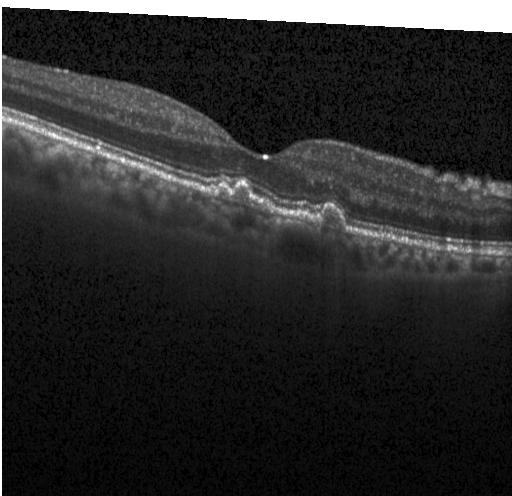

Macular scan, spectral-domain OCT, optical coherence tomography scan, Heidelberg Spectralis OCT system
Dx: drusen.